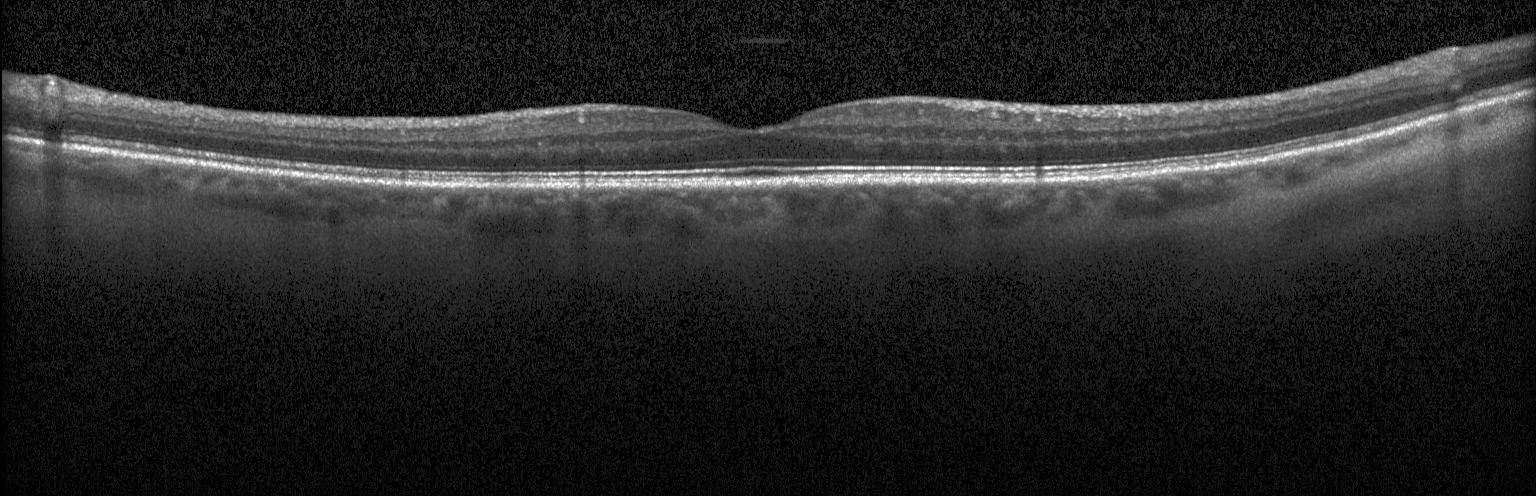 Optical coherence tomography scan, horizontal scan through the fovea, acquired on a Heidelberg Spectralis, spectral-domain OCT
Finding: no evidence of CNV, DME, or drusen.